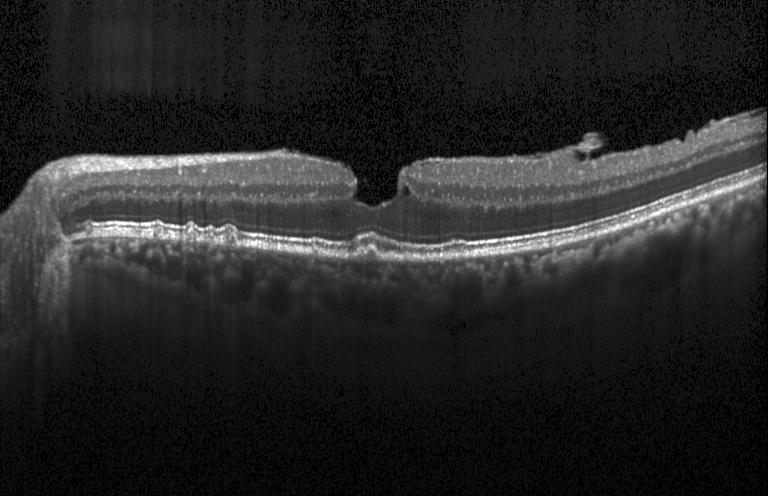

Finding: sub-RPE drusenoid deposits.